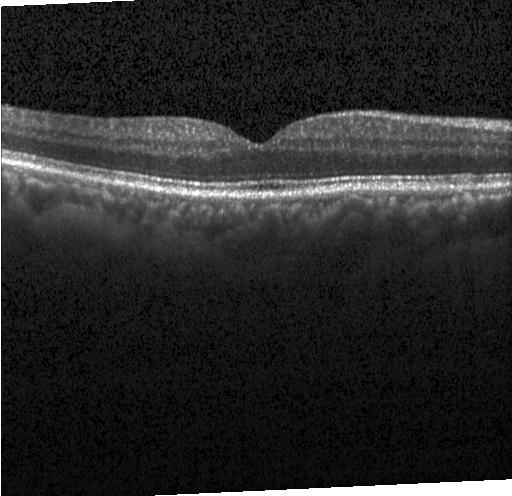

Retinal OCT cross-section · SD-OCT · horizontal scan through the fovea.
Finding: neither CNV, DME, nor drusen.